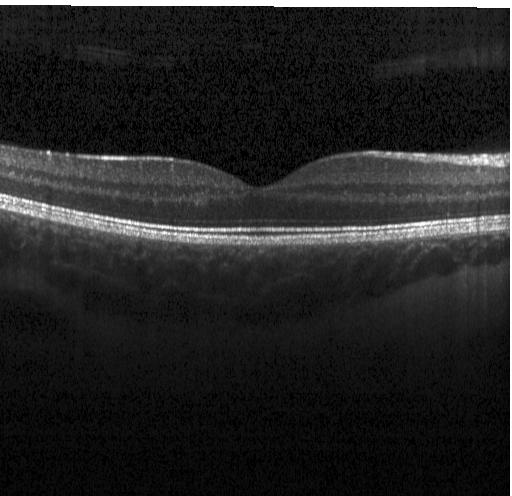

OCT line scan. Macular scan. Finding: no choroidal neovascularization, no diabetic macular edema, and no drusen.